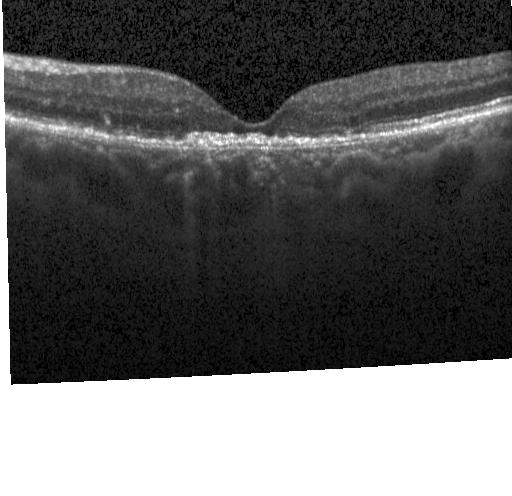
Fovea-centered. Optical coherence tomography B-scan. Spectral-domain optical coherence tomography. Instrument: Heidelberg Spectralis.
Diagnosis: a choroidal neovascular membrane.